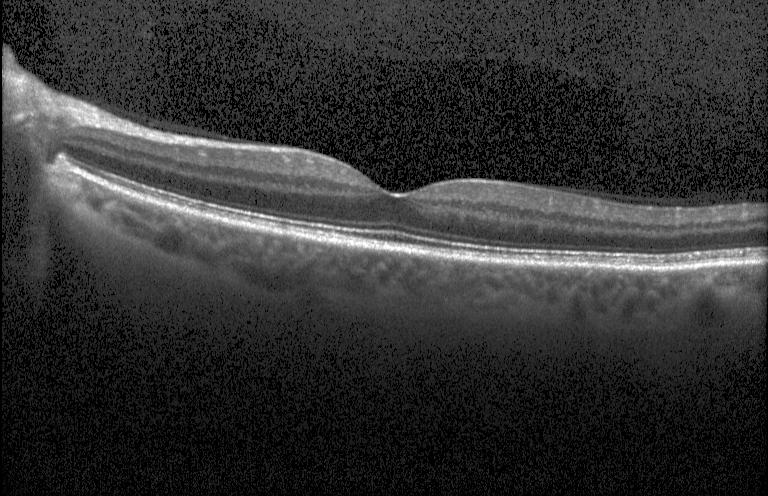 OCT B-scan. Macular OCT: no evidence of CNV, DME, or drusen.